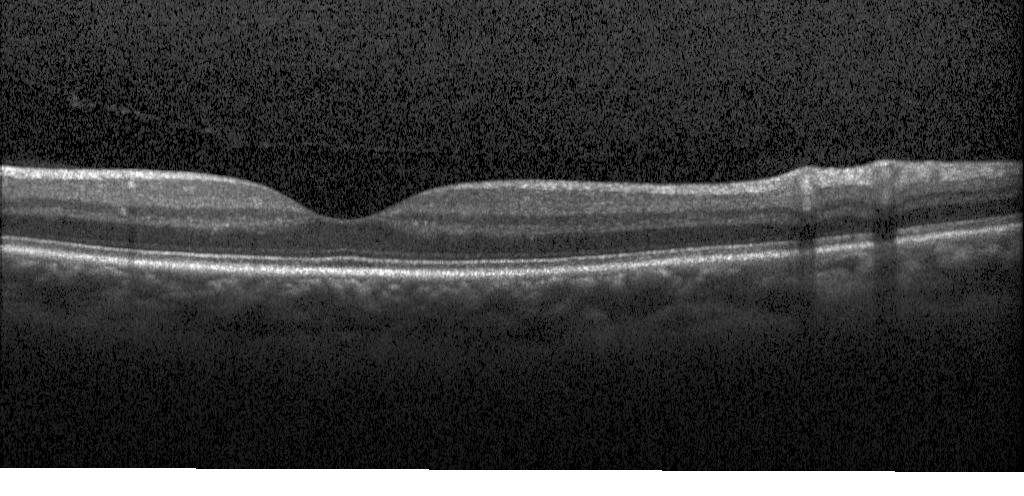
Macular OCT: no choroidal neovascularization, no diabetic macular edema, and no drusen.